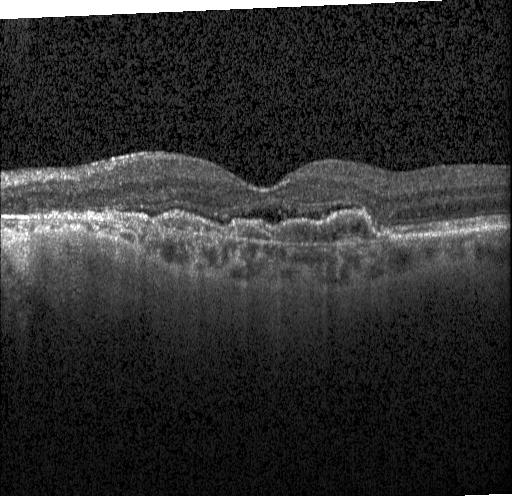

Macular OCT: choroidal neovascularization.